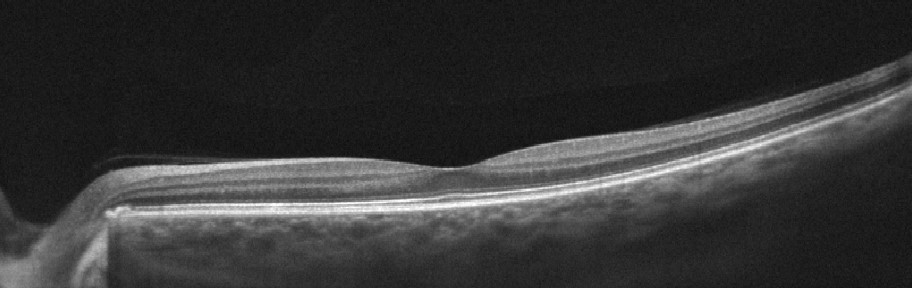

Finding: no AMD, DME, ERM, RAO, RVO, or VID.